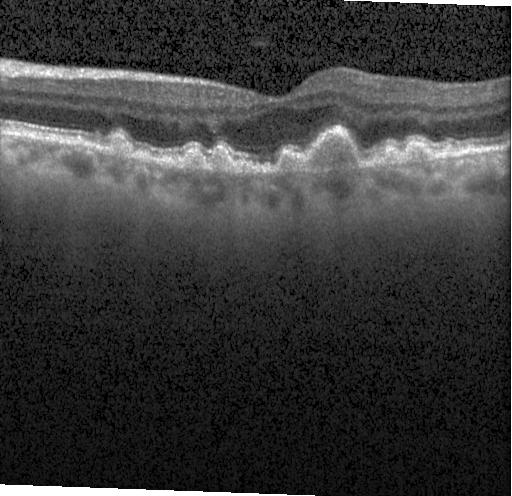
SD-OCT. Centered on the fovea. OCT line scan. Instrument: Heidelberg Spectralis
Assessment: sub-RPE drusenoid deposits.